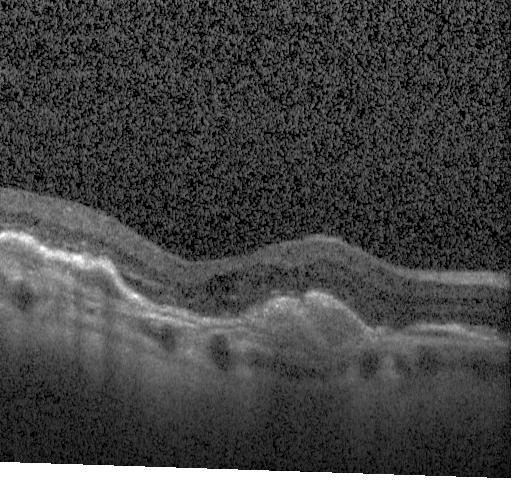 Optical coherence tomography B-scan.
Impression: a choroidal neovascular membrane.